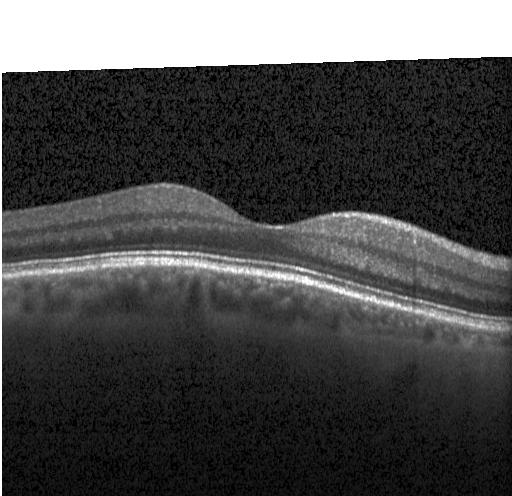
Finding: no evidence of CNV, DME, or drusen.